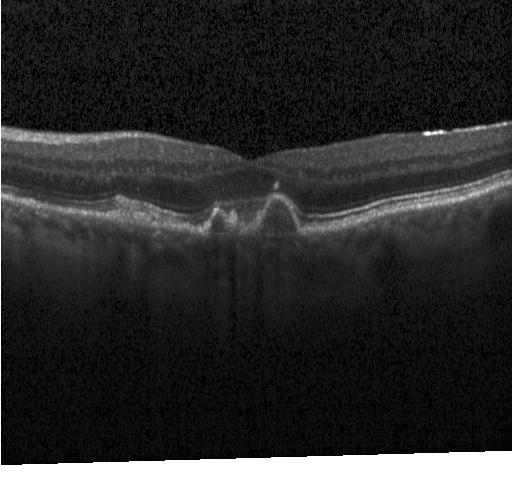

Spectral-domain OCT, Heidelberg Spectralis OCT system, through the macula, optical coherence tomography scan.
OCT finding: CNV.